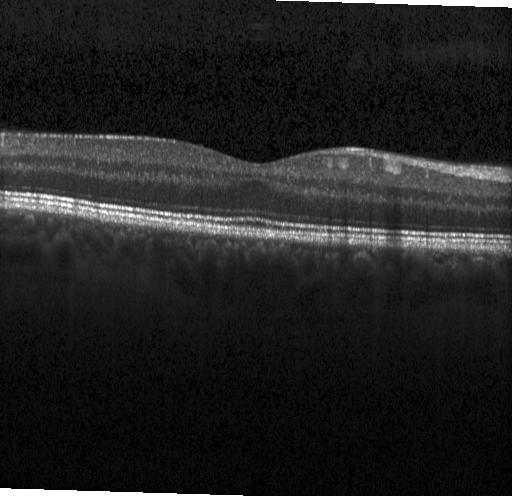

OCT line scan. Spectral-domain optical coherence tomography — The scan shows neither choroidal neovascularization, diabetic macular edema, nor drusen.